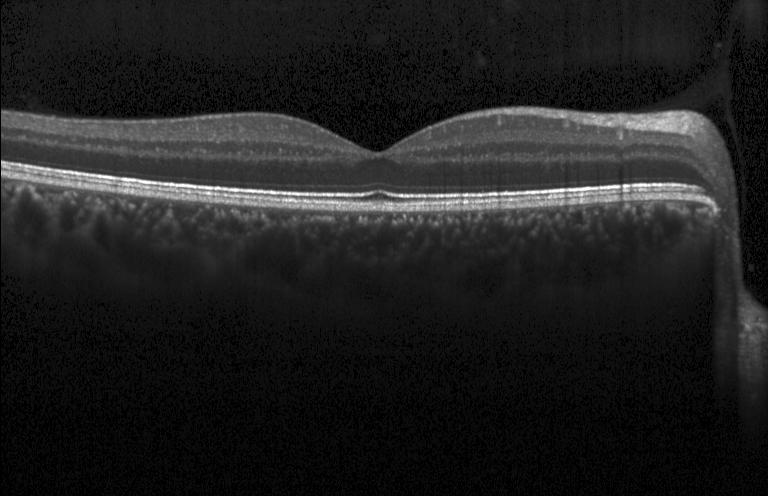

Retinal OCT B-scan.
Dx: no CNV, DME, or drusen.